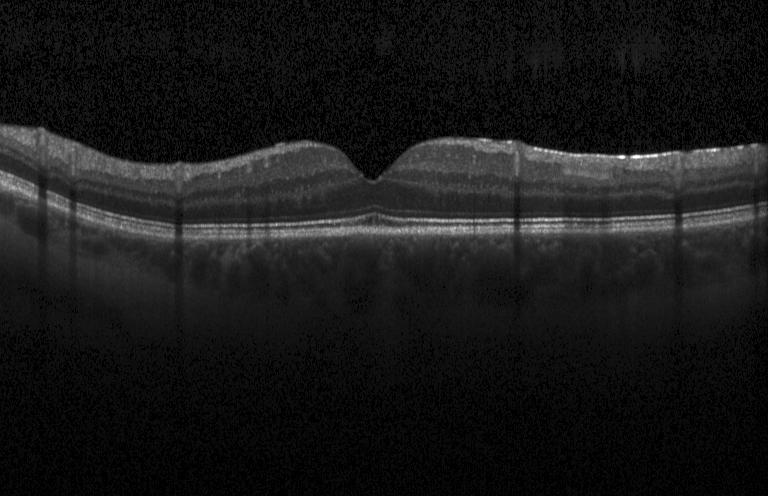

Retinal OCT B-scan. Fovea-centered. Instrument: Heidelberg Spectralis
Diagnosis: no choroidal neovascularization, no diabetic macular edema, and no drusen.